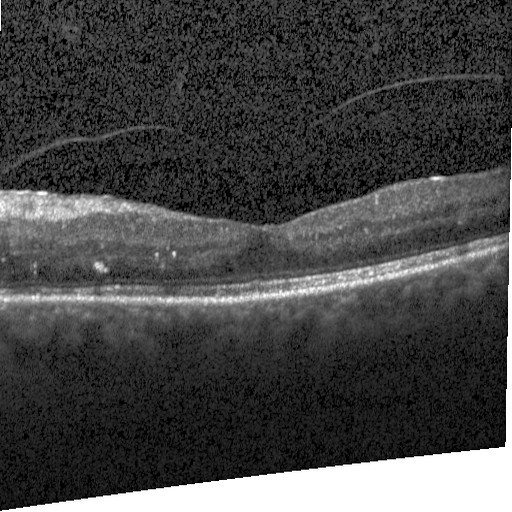 OCT line scan
Impression: DME.